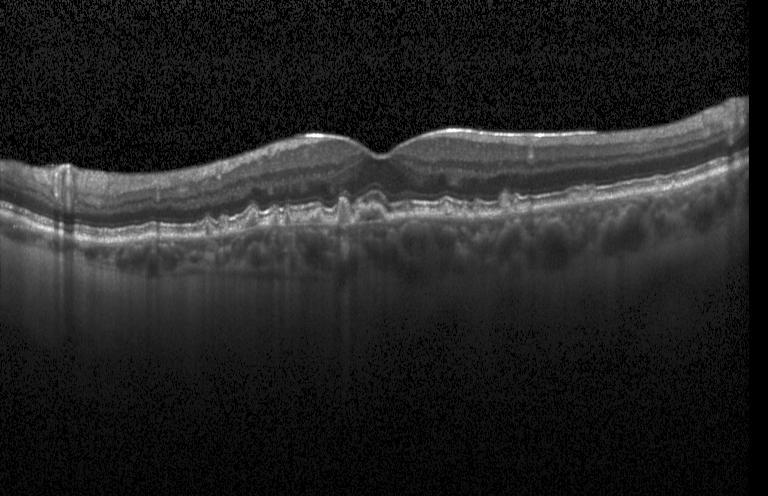 Retinal OCT B-scan.
Diagnosis: sub-RPE drusenoid deposits.